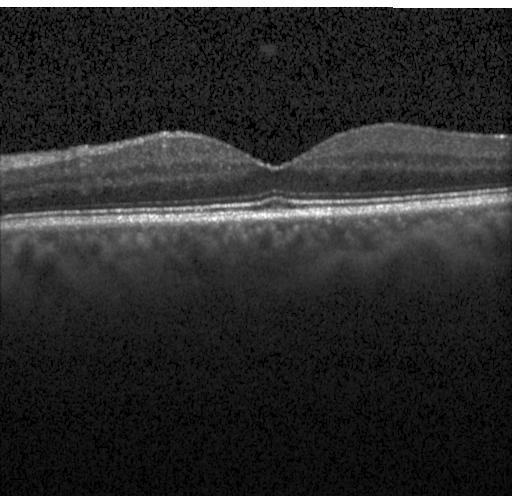

Heidelberg Spectralis, optical coherence tomography scan.
Impression: no choroidal neovascularization, no diabetic macular edema, and no drusen.